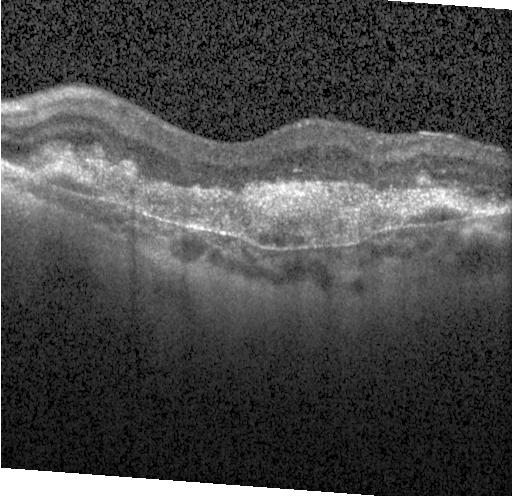

Macular scan. OCT line scan. Heidelberg Spectralis. SD-OCT — Impression: a choroidal neovascular membrane.